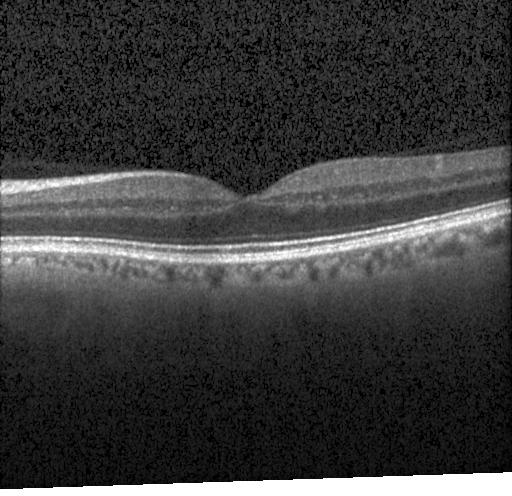

OCT B-scan showing no choroidal neovascularization, diabetic macular edema, or drusen.